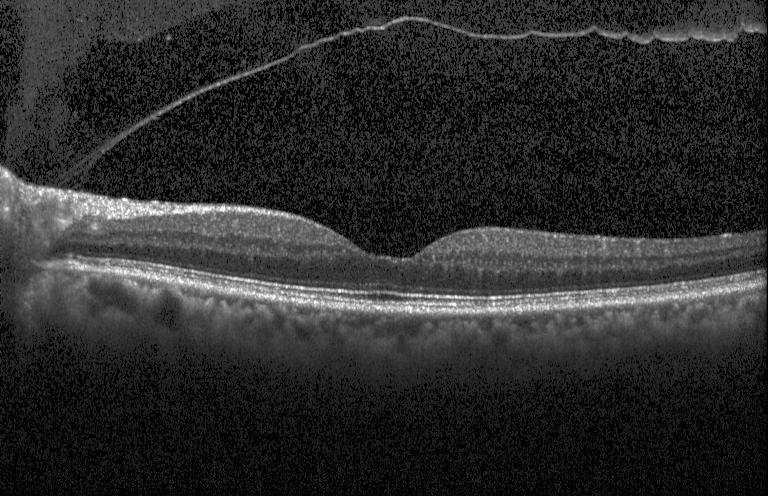 OCT B-scan. Impression: no evidence of choroidal neovascularization, diabetic macular edema, or drusen.